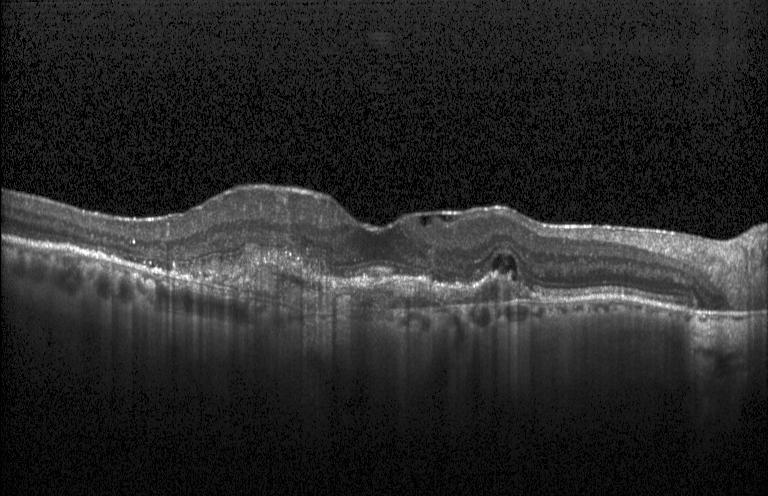

Horizontal scan through the fovea; acquired on a Heidelberg Spectralis; OCT line scan.
Finding: choroidal neovascularization.